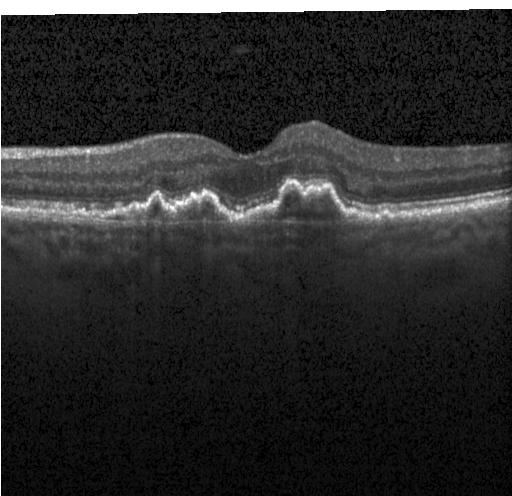 Macular OCT demonstrating a choroidal neovascular membrane.